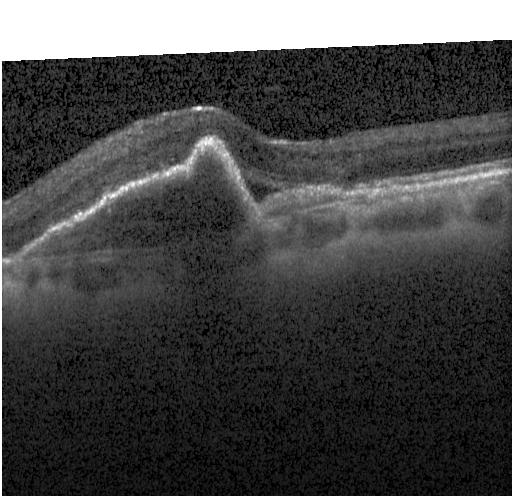
Diagnosis: choroidal neovascularization (CNV).